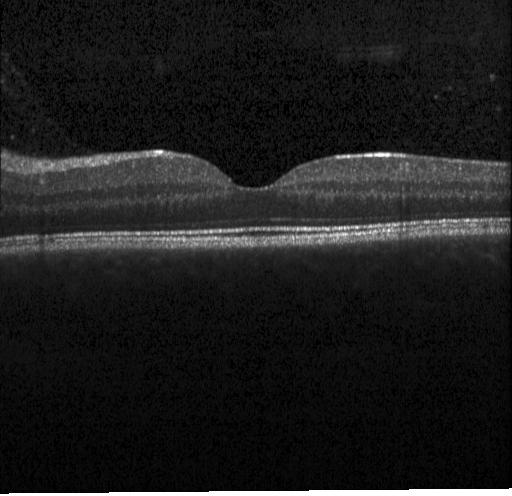

Diagnosis: no choroidal neovascularization, diabetic macular edema, or drusen.